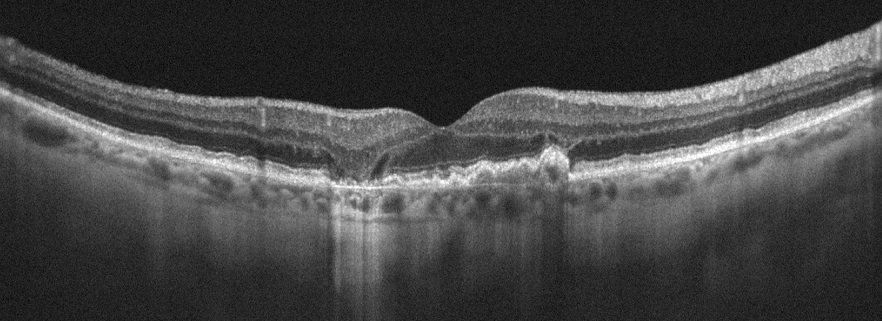

OCT finding: AMD.